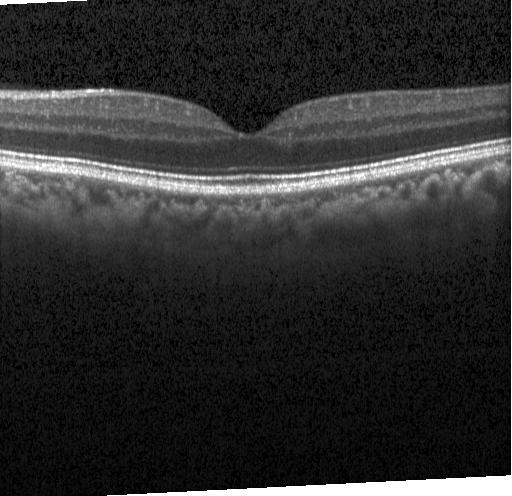
Diagnosis: no evidence of choroidal neovascularization, diabetic macular edema, or drusen.